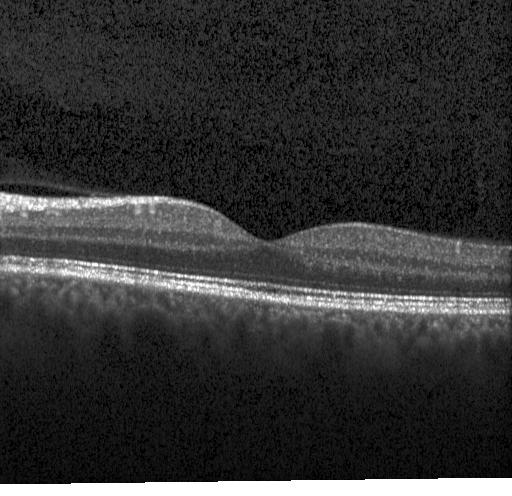

OCT B-scan showing no evidence of choroidal neovascularization, diabetic macular edema, or drusen.